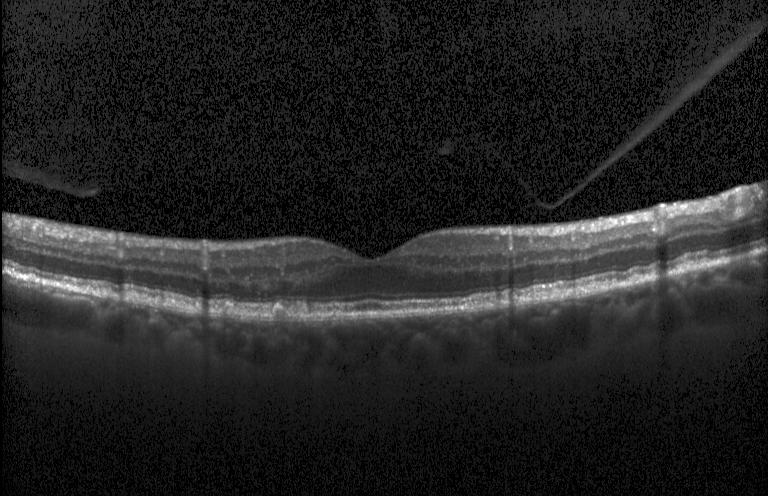
OCT finding: multiple drusen.